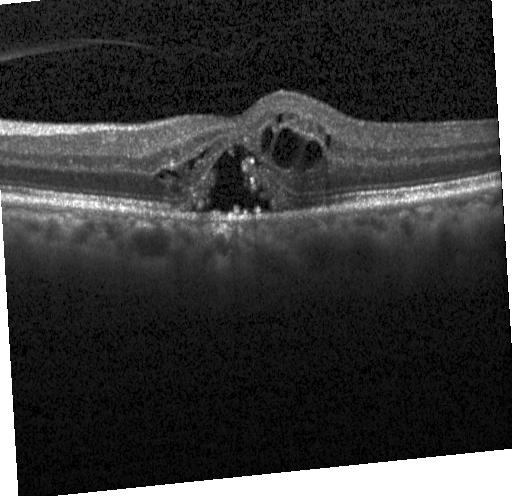 The scan shows a choroidal neovascular membrane.